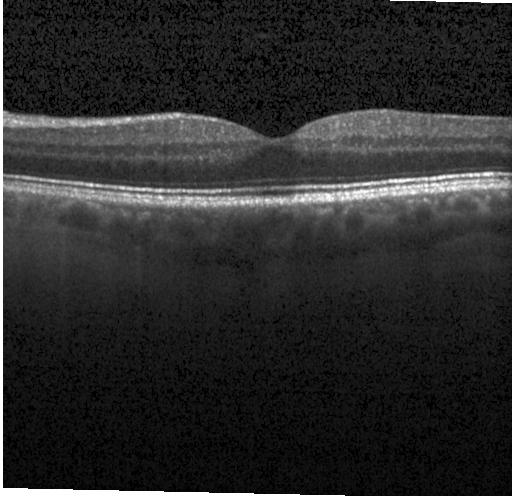
SD-OCT. Retinal OCT B-scan. Heidelberg Spectralis.
No choroidal neovascularization, no diabetic macular edema, and no drusen.